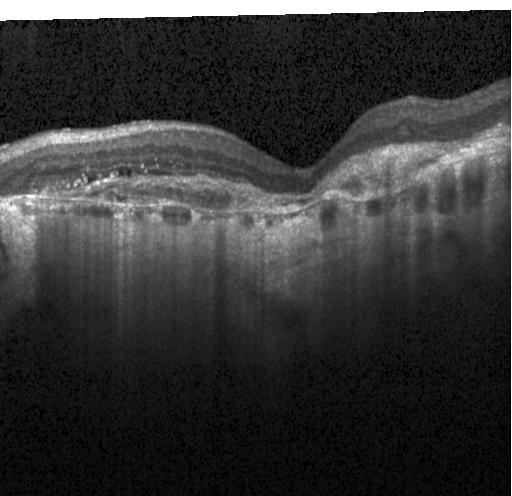

Retinal OCT B-scan; Heidelberg Spectralis OCT system; horizontal scan through the fovea; spectral-domain OCT. This B-scan demonstrates choroidal neovascularization.